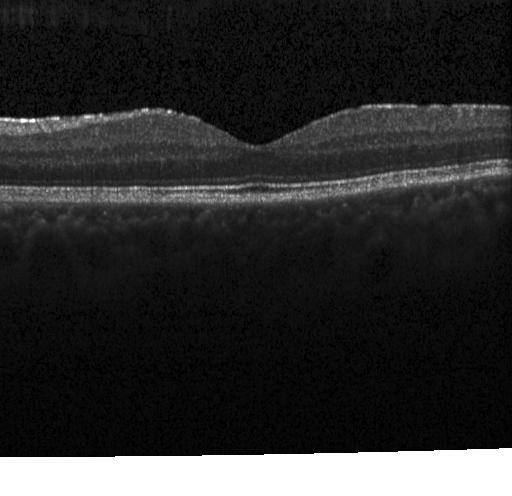 SD-OCT · optical coherence tomography scan. OCT finding: neither CNV, DME, nor drusen.